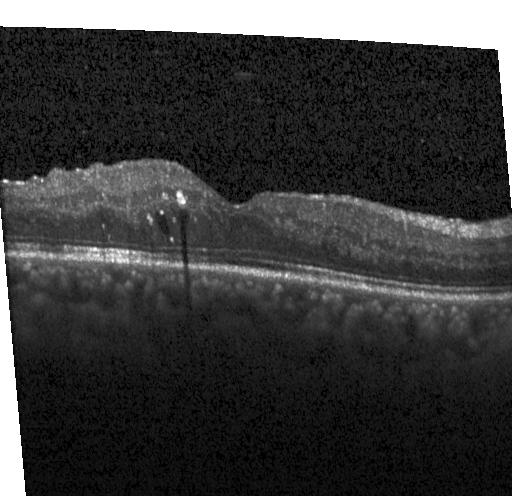
Optical coherence tomography B-scan.
Diabetic macular edema.